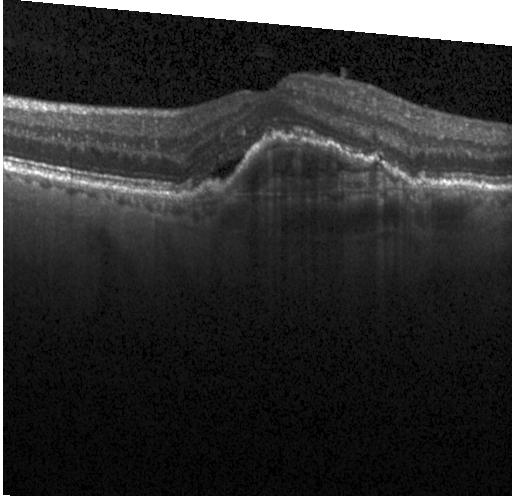

Optical coherence tomography scan.
Diagnosis: choroidal neovascularization (CNV).